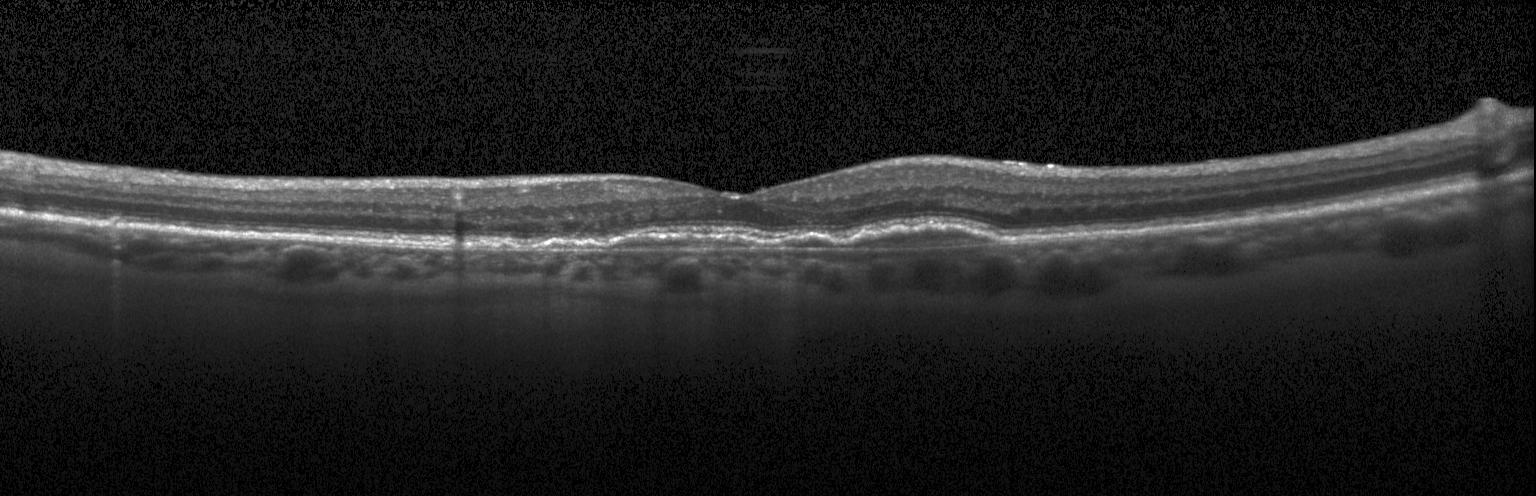

Retinal OCT cross-section showing choroidal neovascularization (CNV).